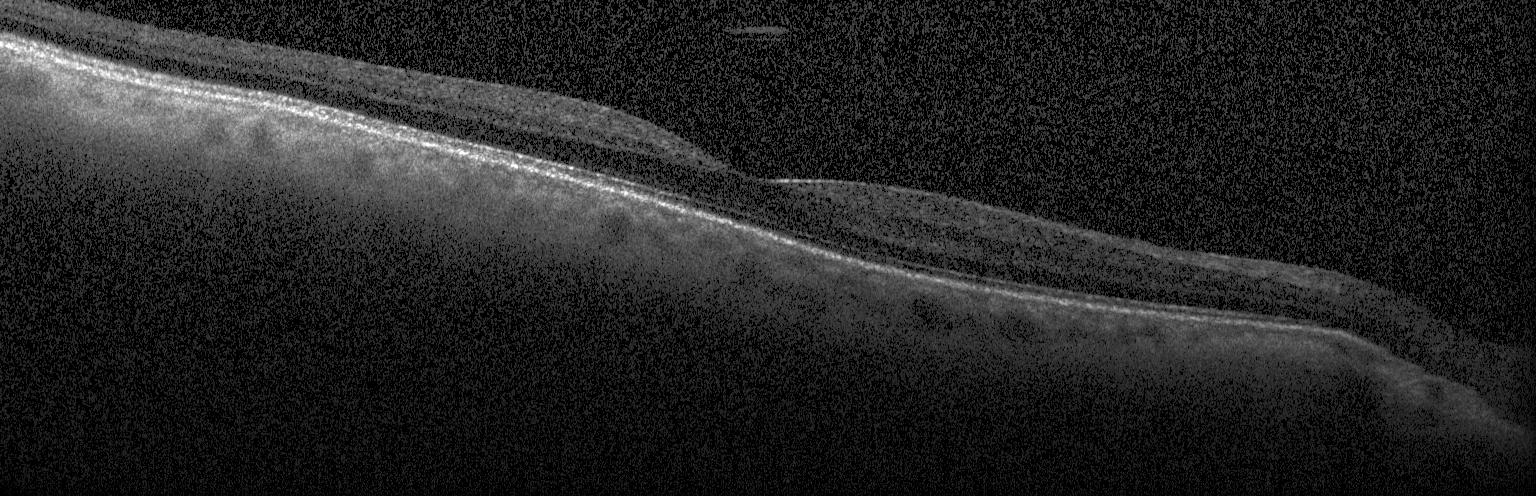

No CNV, DME, or drusen.